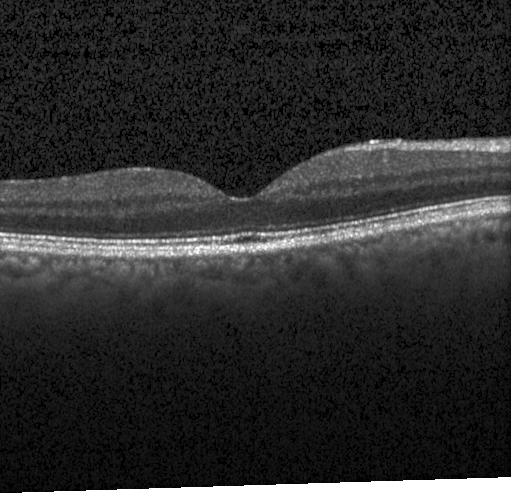
Retinal OCT B-scan · macular scan.
Finding: no choroidal neovascularization, diabetic macular edema, or drusen.